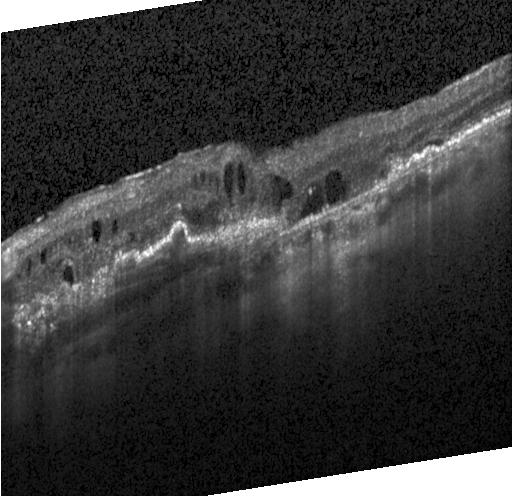
OCT B-scan · through the macula.
Assessment: a choroidal neovascular membrane.